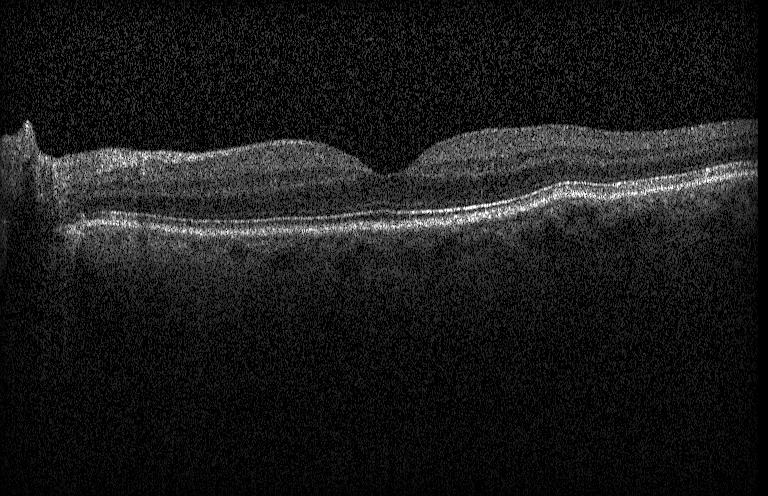
OCT line scan. Centered on the fovea. Heidelberg Spectralis.
Finding: no CNV, DME, or drusen.